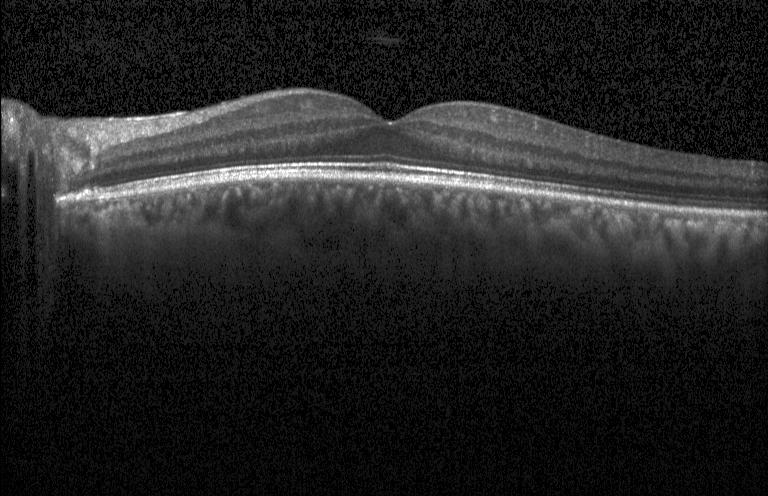 Retinal OCT B-scan. Spectral-domain optical coherence tomography — Assessment: neither choroidal neovascularization, diabetic macular edema, nor drusen.